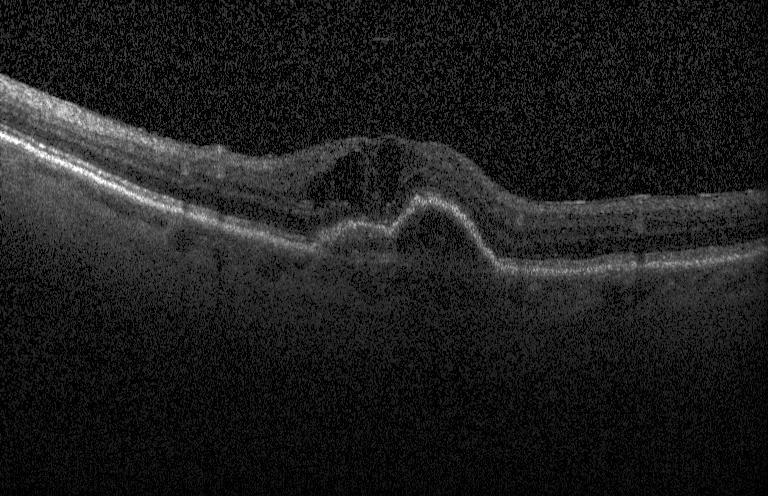

OCT finding: choroidal neovascularization.